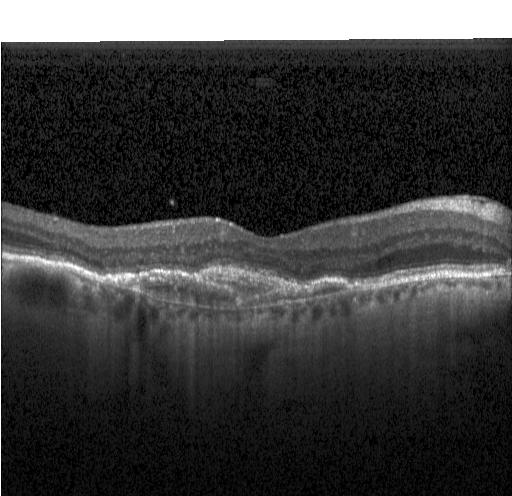
Impression: choroidal neovascularization.